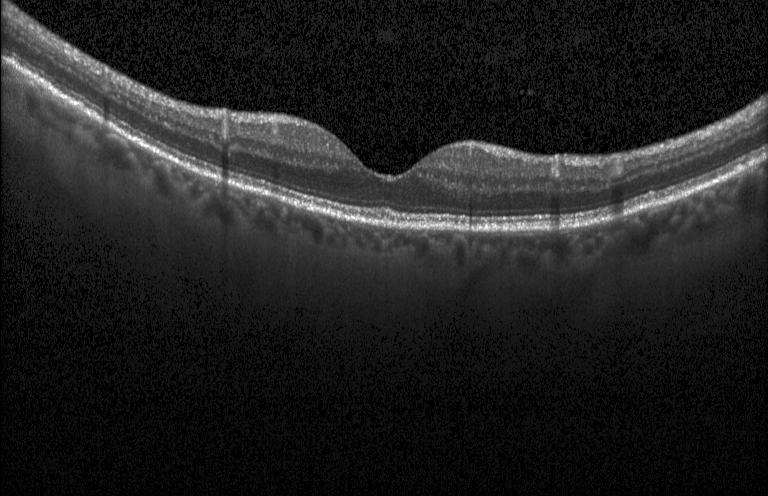 Retinal OCT cross-section.
Diagnosis: neither CNV, DME, nor drusen.